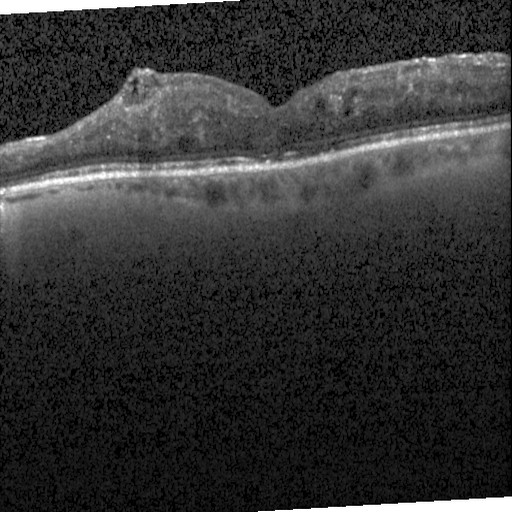

Diagnosis: DME.